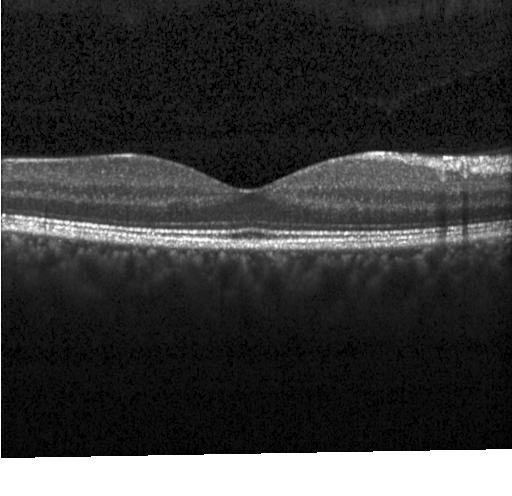 Instrument: Heidelberg Spectralis, macular scan, spectral-domain OCT, OCT line scan — Diagnosis: neither choroidal neovascularization, diabetic macular edema, nor drusen.